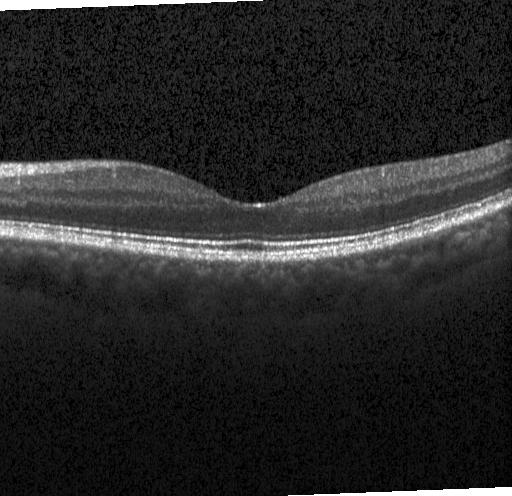

Optical coherence tomography B-scan, Heidelberg Spectralis OCT system.
Impression: neither choroidal neovascularization, diabetic macular edema, nor drusen.